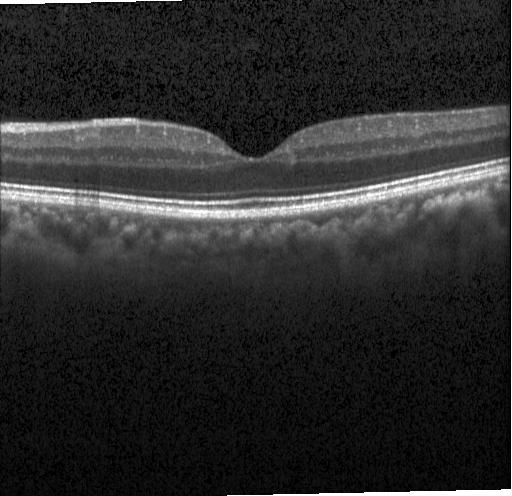
Optical coherence tomography B-scan · spectral-domain optical coherence tomography · through the macula
This B-scan demonstrates neither choroidal neovascularization, diabetic macular edema, nor drusen.